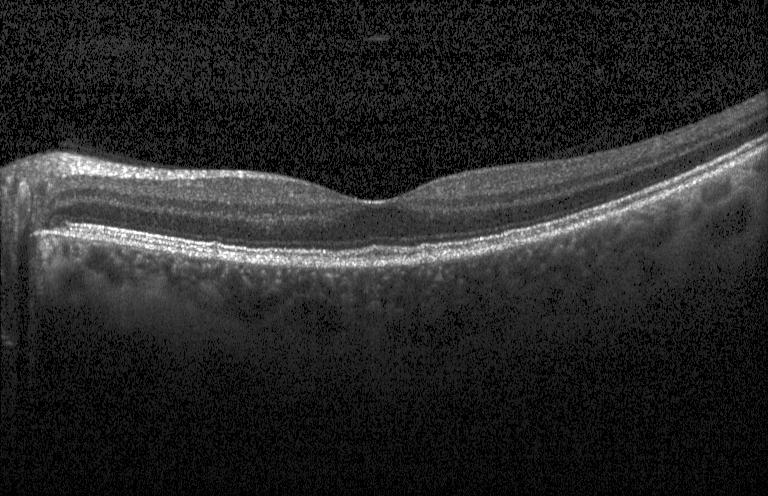
Assessment: neither choroidal neovascularization, diabetic macular edema, nor drusen.